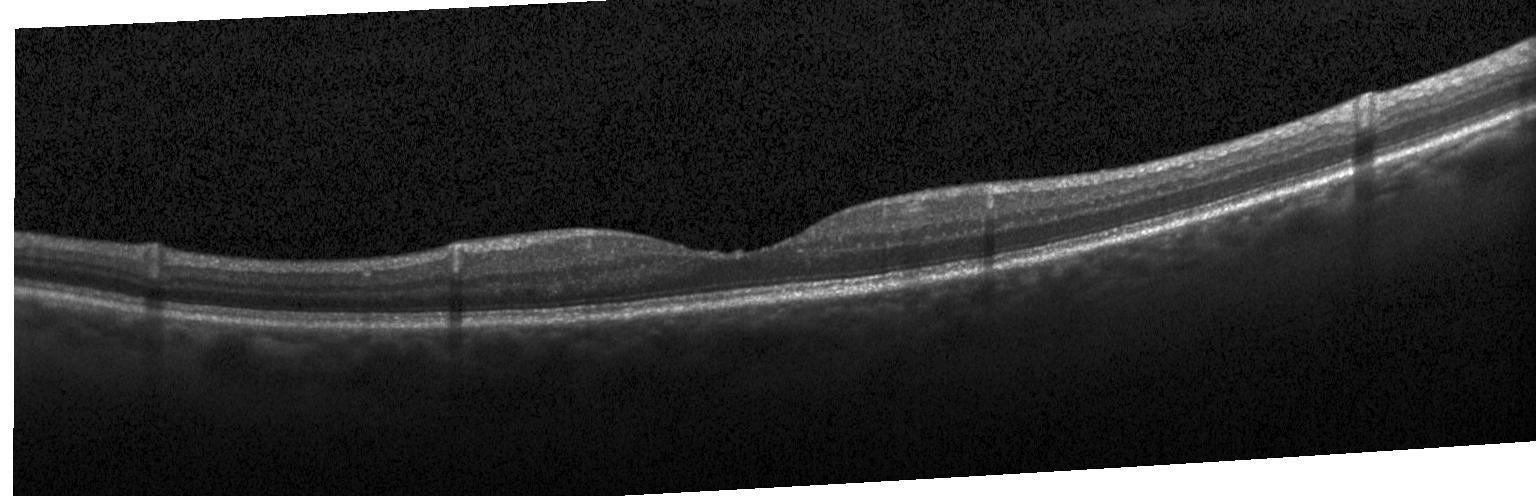
Heidelberg Spectralis OCT system, OCT B-scan — Macular OCT: no choroidal neovascularization, diabetic macular edema, or drusen.